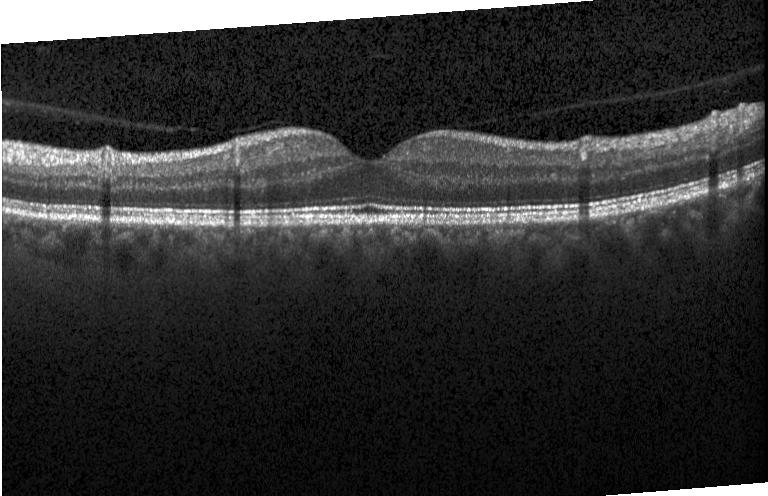 Finding: no choroidal neovascularization, no diabetic macular edema, and no drusen.